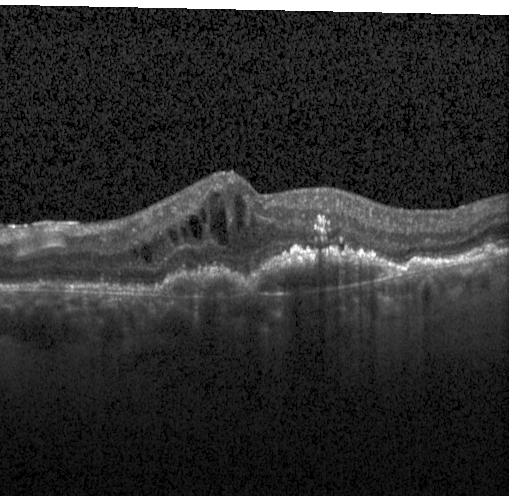
Optical coherence tomography scan · acquired on a Heidelberg Spectralis · SD-OCT.
Finding: choroidal neovascularization.